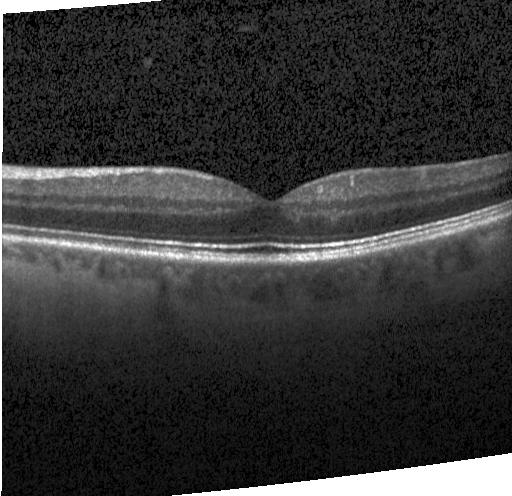 Finding: no evidence of CNV, DME, or drusen.